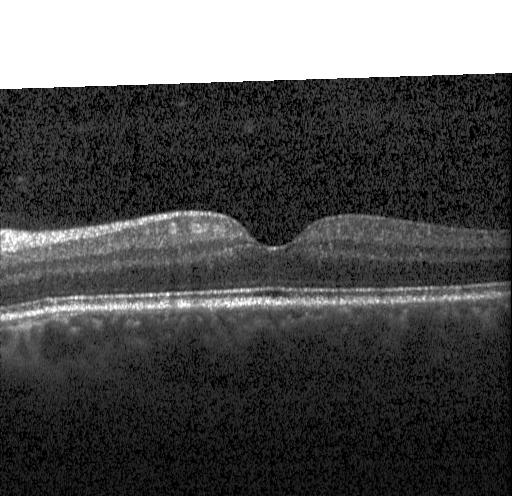
Retinal OCT B-scan · SD-OCT.
Finding: no choroidal neovascularization, diabetic macular edema, or drusen.